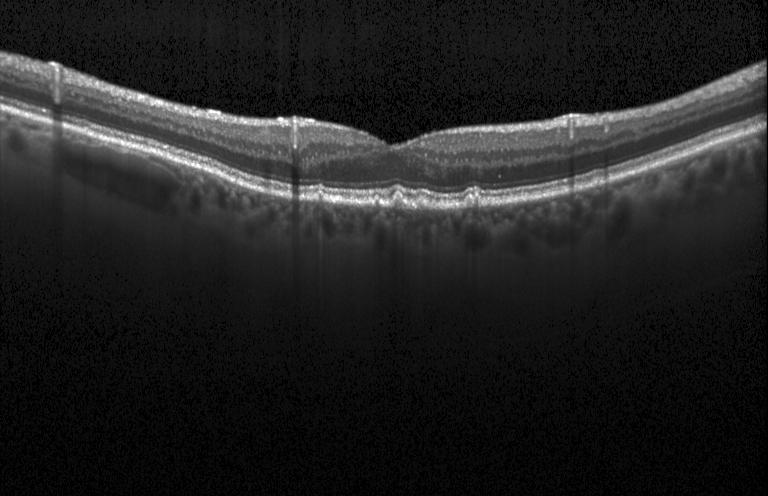

Impression: multiple drusen.